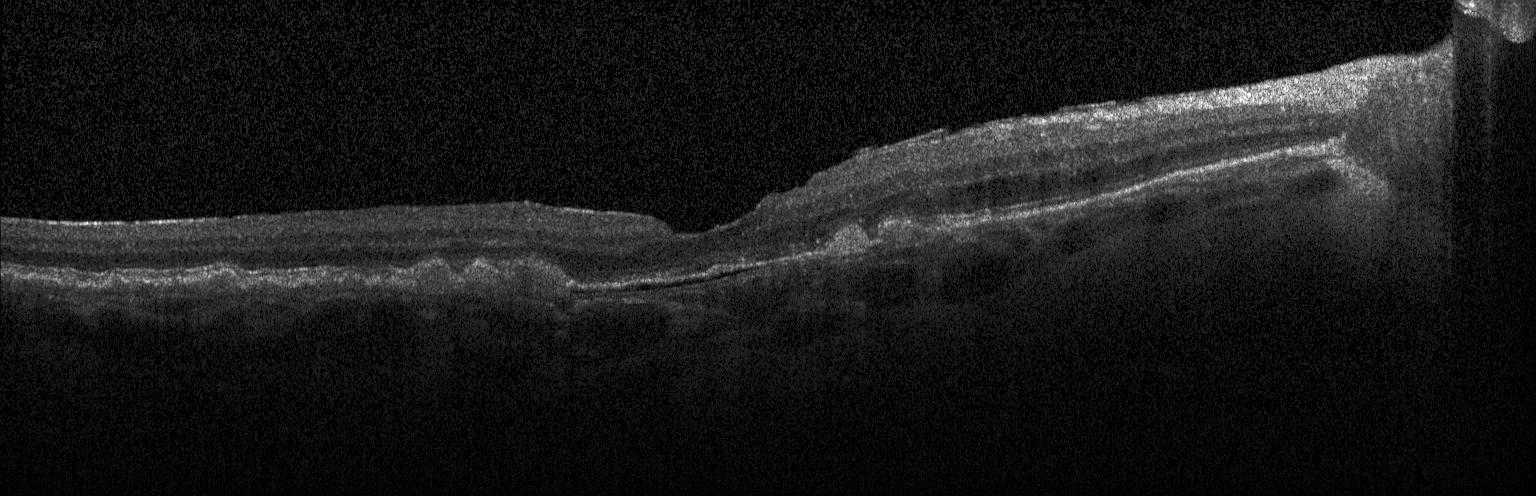

Impression: a choroidal neovascular membrane.